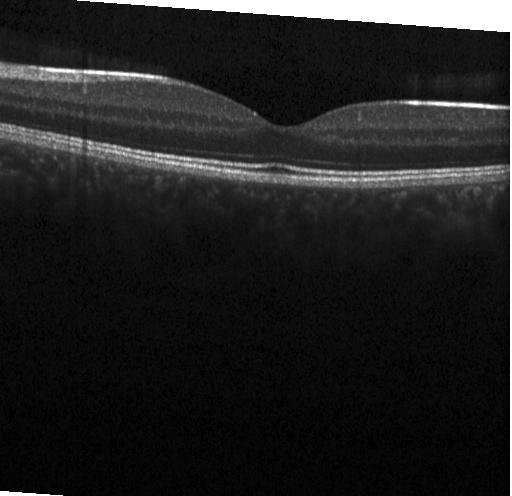

Spectral-domain OCT, OCT B-scan.
OCT finding: no choroidal neovascularization, diabetic macular edema, or drusen.